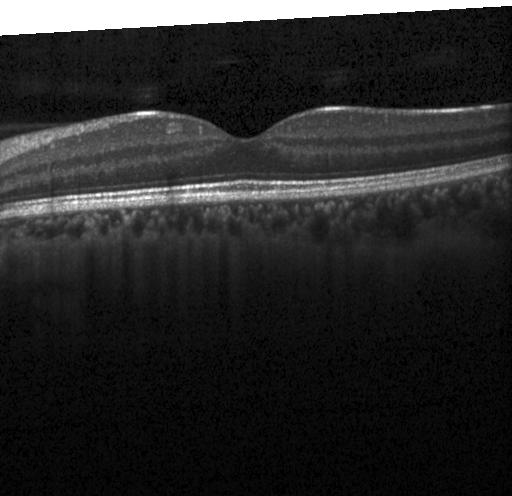 Assessment: neither choroidal neovascularization, diabetic macular edema, nor drusen.